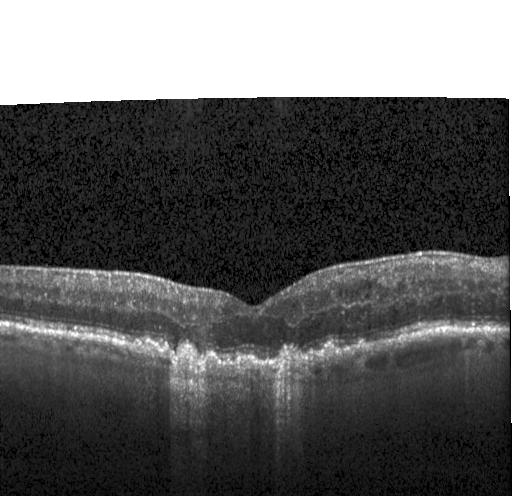

Assessment: a choroidal neovascular membrane.